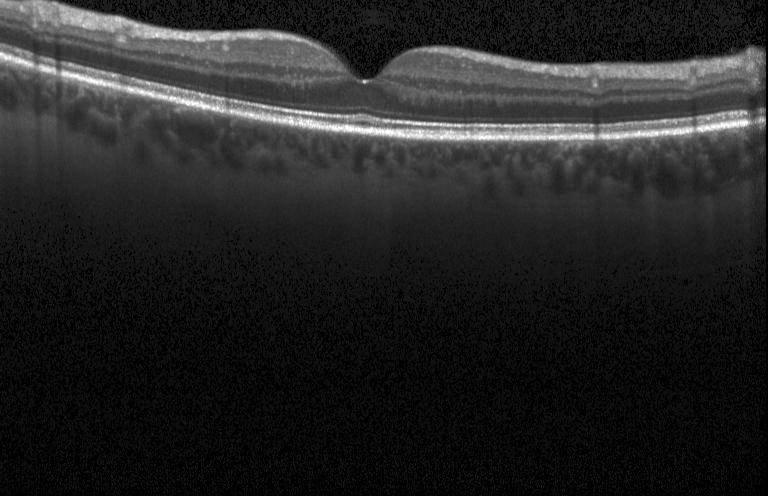

Assessment: no evidence of choroidal neovascularization, diabetic macular edema, or drusen.